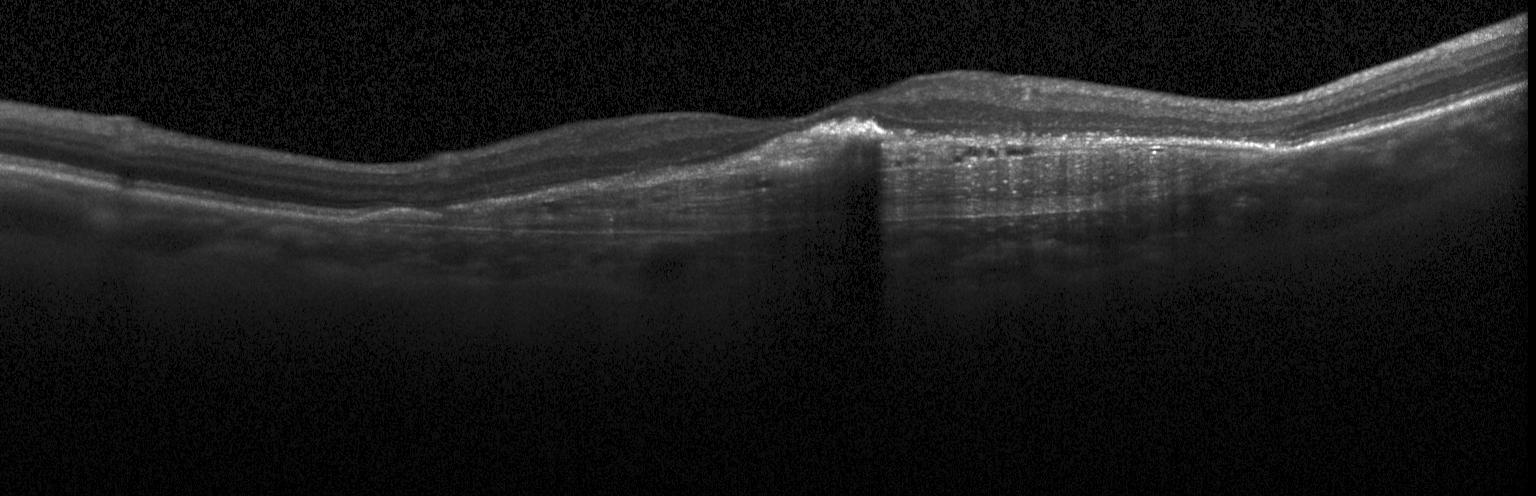 A choroidal neovascular membrane.